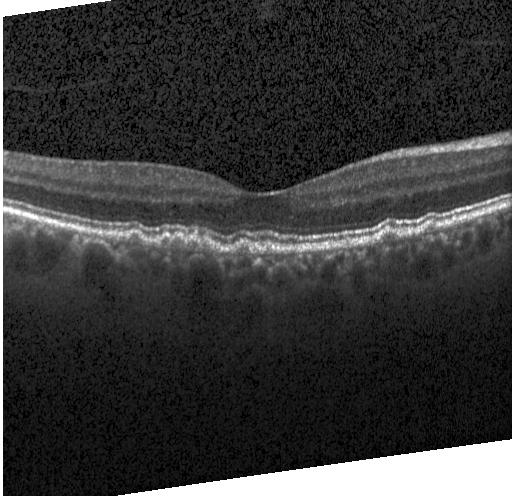
Spectral-domain OCT. Centered on the fovea. Acquired on a Heidelberg Spectralis. OCT line scan. Macular OCT: drusen.